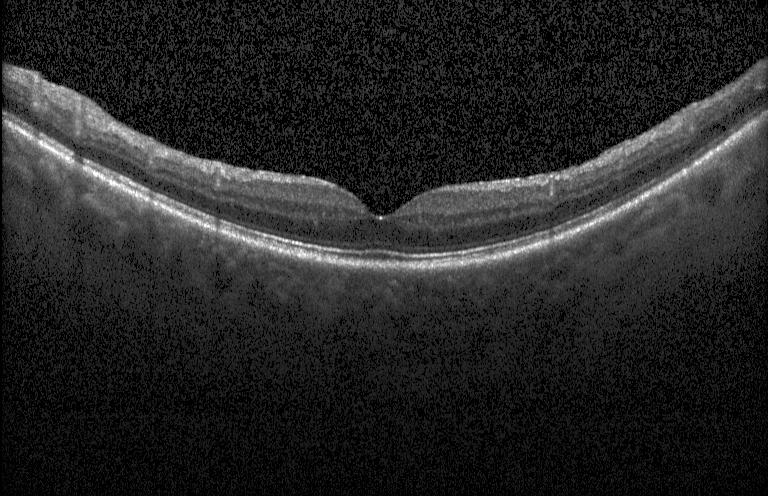

OCT scan showing no choroidal neovascularization, no diabetic macular edema, and no drusen.